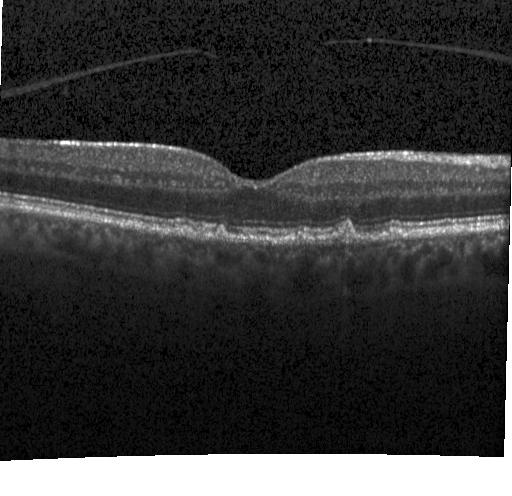 Retinal OCT cross-section showing drusen.